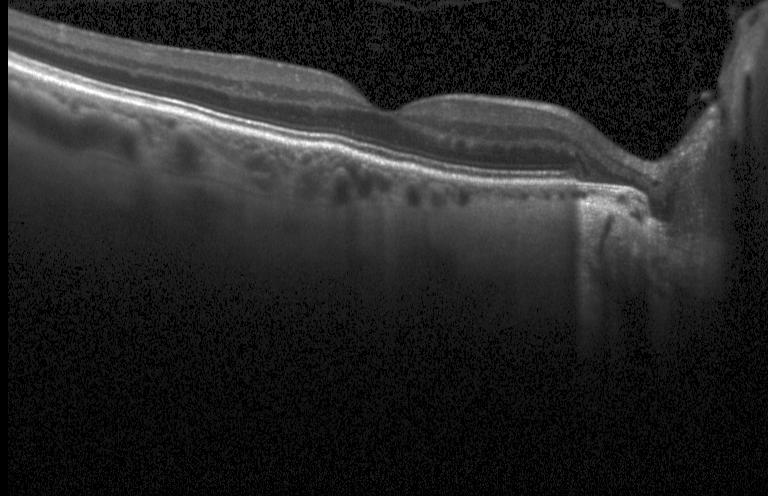 Dx: no evidence of CNV, DME, or drusen.